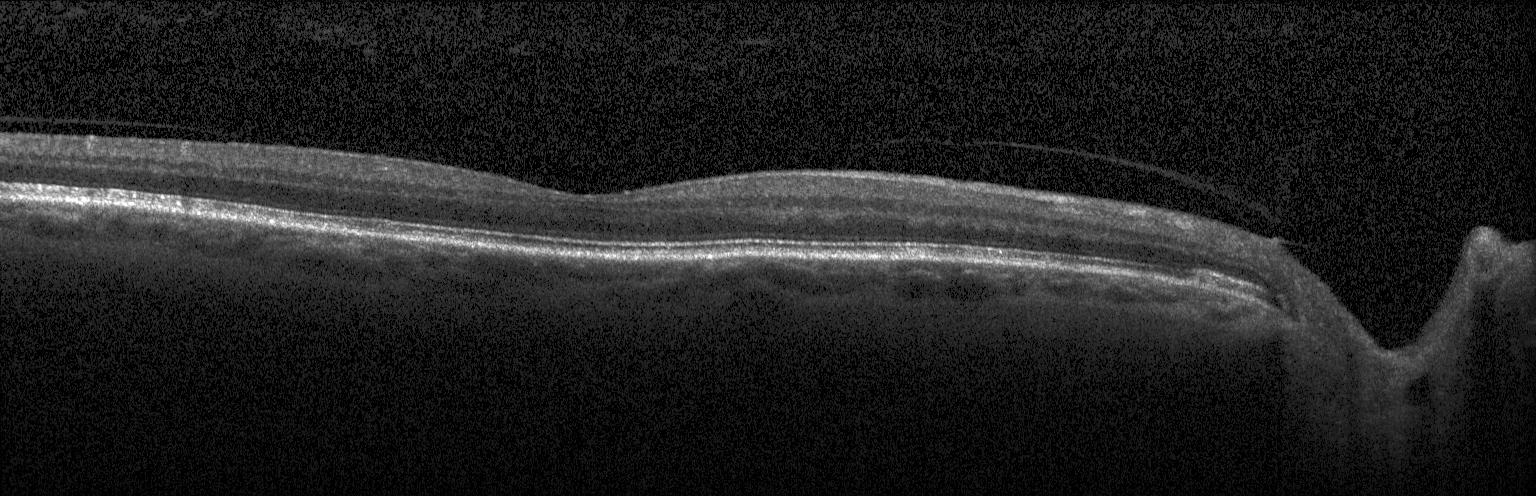 OCT line scan. Acquired on a Heidelberg Spectralis. Spectral-domain OCT. Dx: no CNV, DME, or drusen.